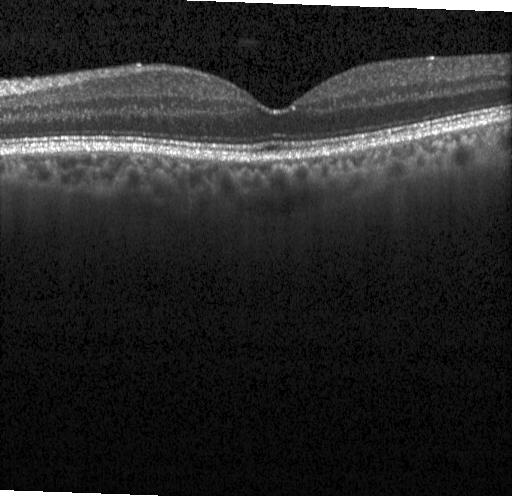

Optical coherence tomography scan. Dx: no choroidal neovascularization, diabetic macular edema, or drusen.